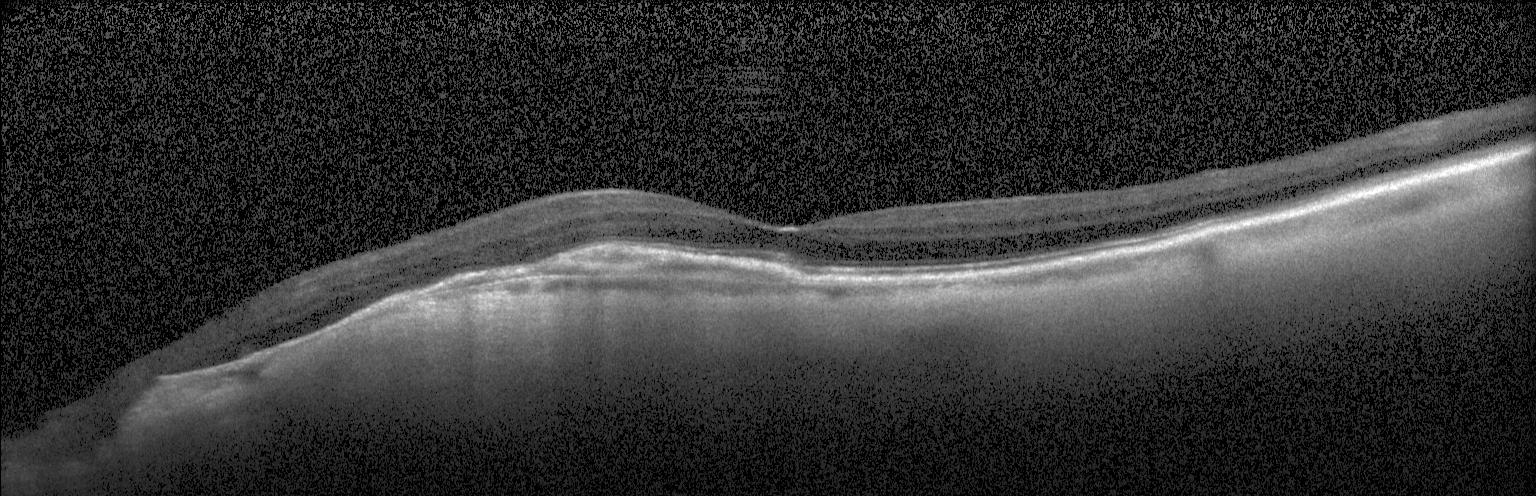 OCT line scan. Impression: choroidal neovascularization (CNV).